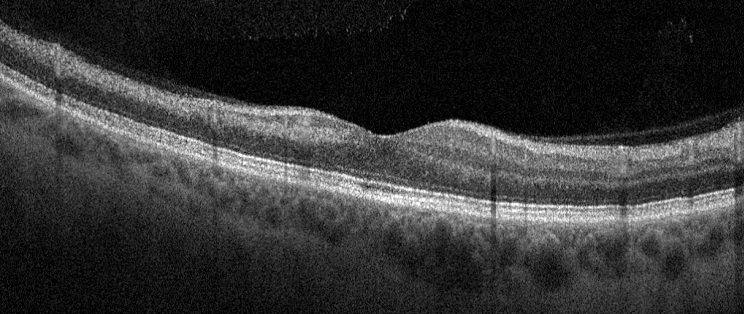

Retinal OCT B-scan. Impression: retinal vein occlusion (RVO).